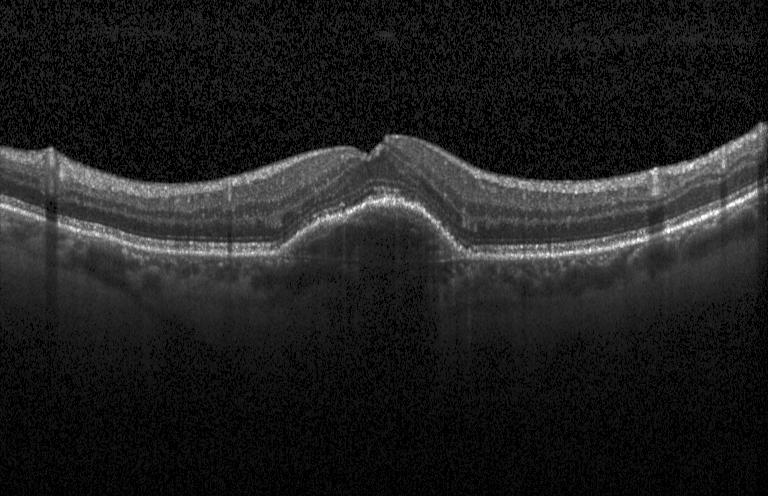 OCT line scan. Acquired on a Heidelberg Spectralis — Assessment: CNV.